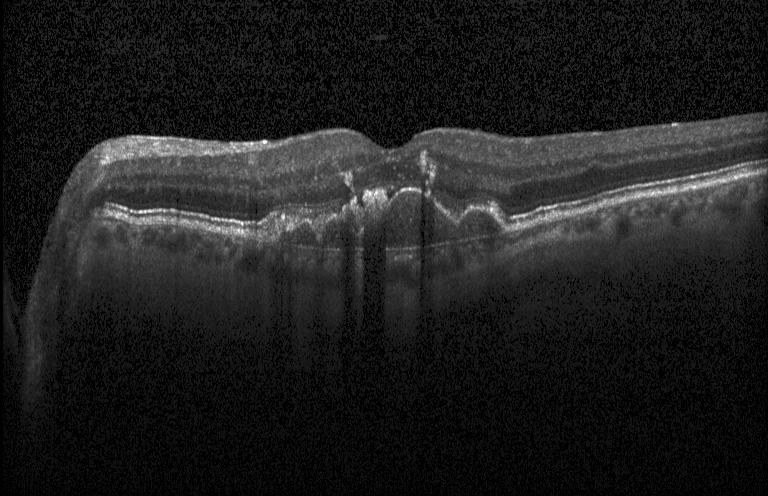 Finding: a choroidal neovascular membrane.